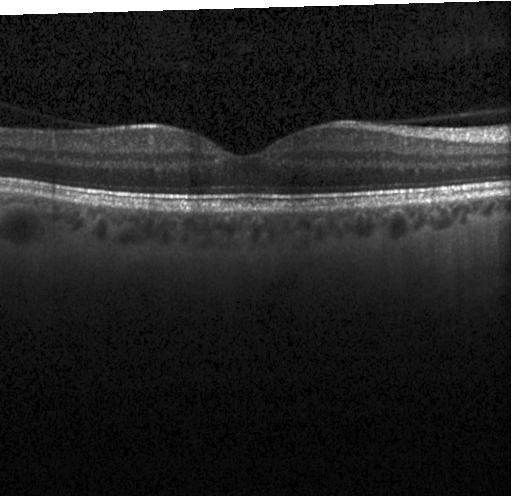

Retinal OCT cross-section · spectral-domain OCT.
This B-scan demonstrates no evidence of choroidal neovascularization, diabetic macular edema, or drusen.